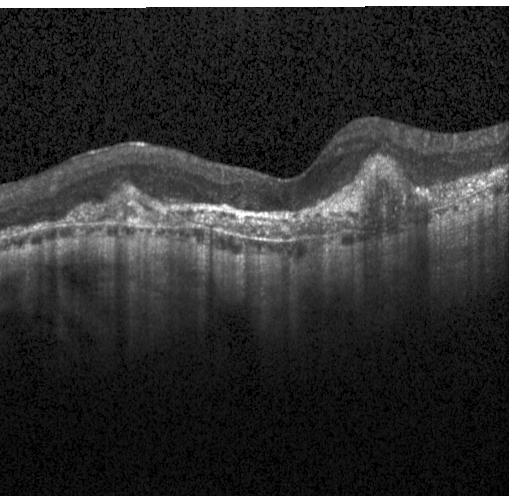
OCT B-scan; SD-OCT — This B-scan demonstrates a choroidal neovascular membrane.